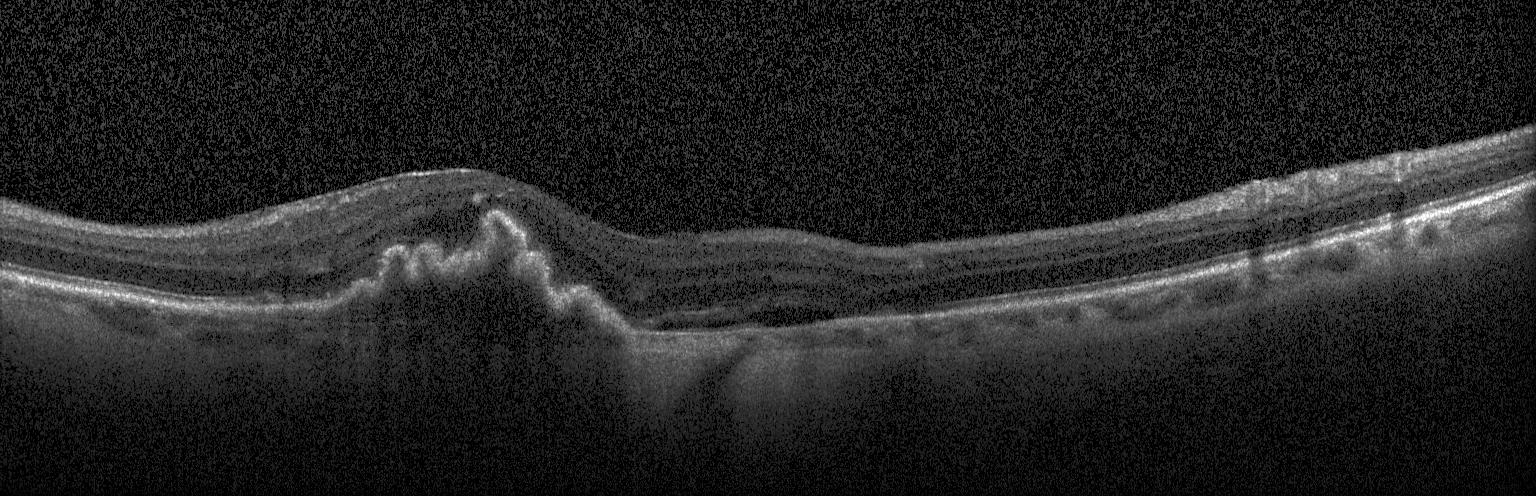 Impression: CNV.